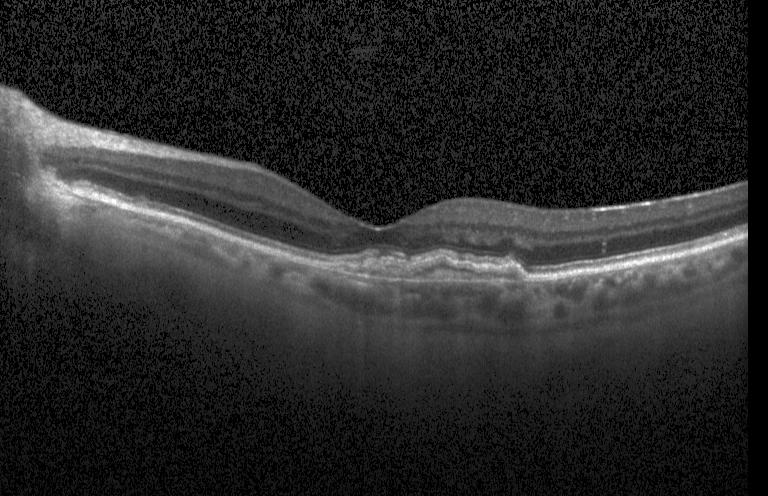
Optical coherence tomography B-scan. Diagnosis: choroidal neovascularization.